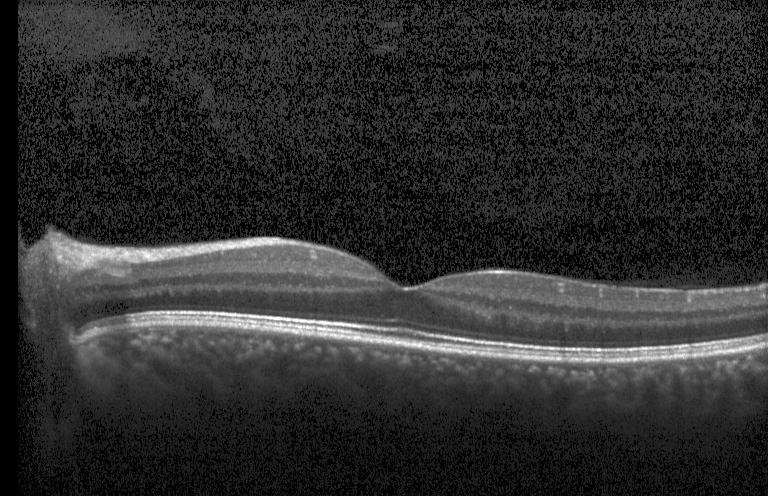
Retinal OCT cross-section showing neither CNV, DME, nor drusen.